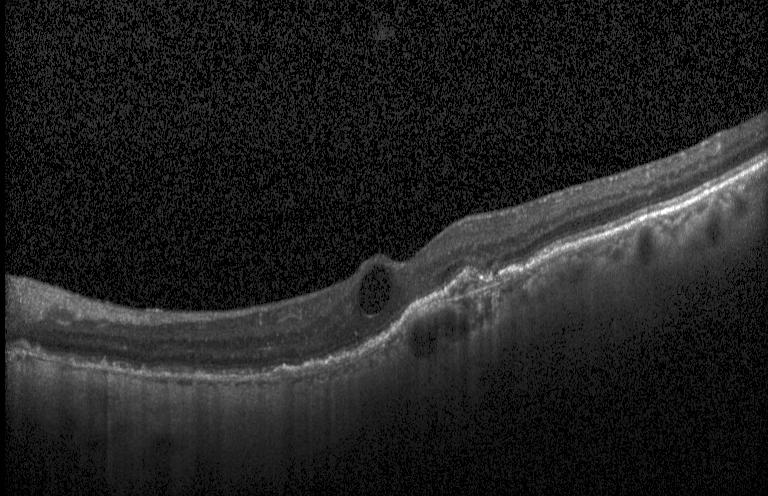 Impression: a choroidal neovascular membrane.